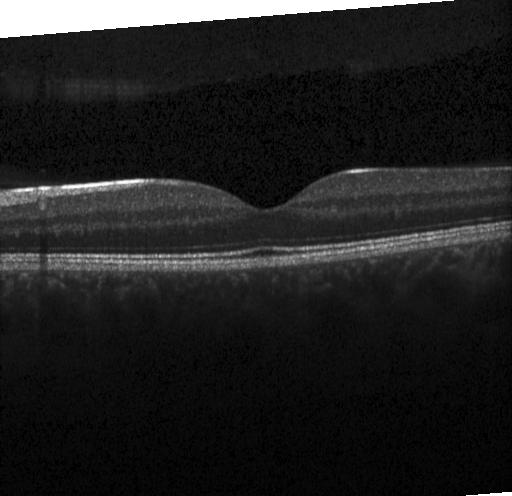

Finding: no choroidal neovascularization, no diabetic macular edema, and no drusen.